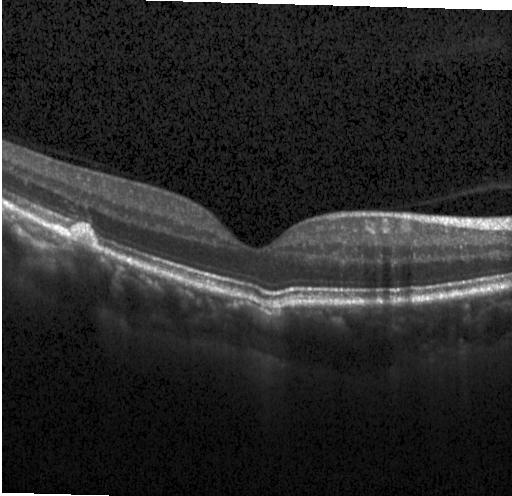

Instrument: Heidelberg Spectralis; spectral-domain OCT; retinal OCT cross-section; fovea-centered
Finding: drusen.